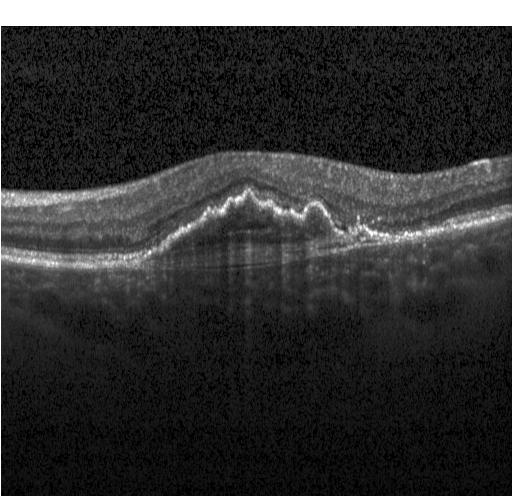

The scan shows choroidal neovascularization.